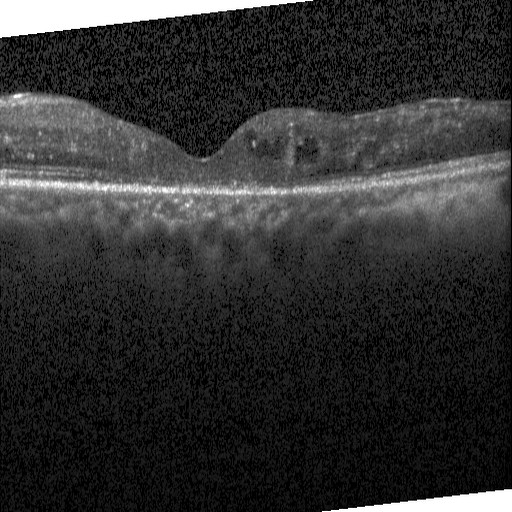

Retinal OCT B-scan · through the macula · instrument: Heidelberg Spectralis. Finding: DME.